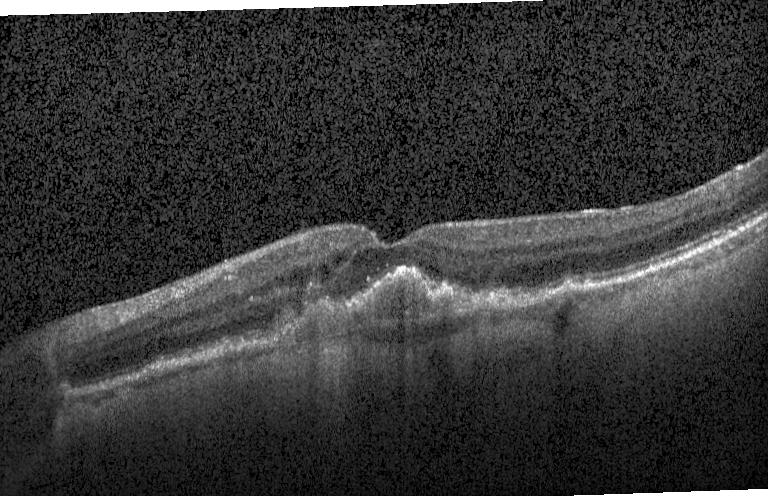 Optical coherence tomography scan · acquired on a Heidelberg Spectralis · spectral-domain optical coherence tomography · through the macula
Dx: choroidal neovascularization (CNV).